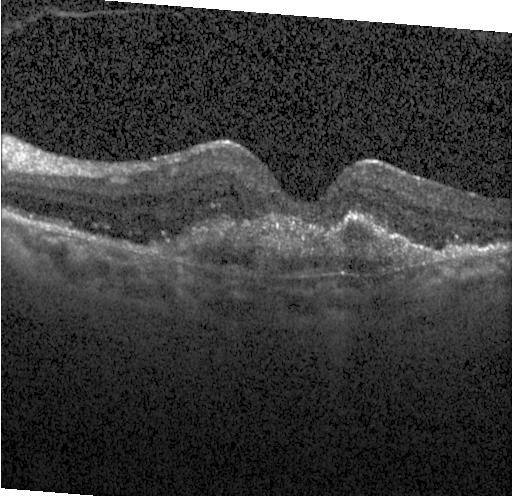
OCT B-scan.
Assessment: choroidal neovascularization (CNV).